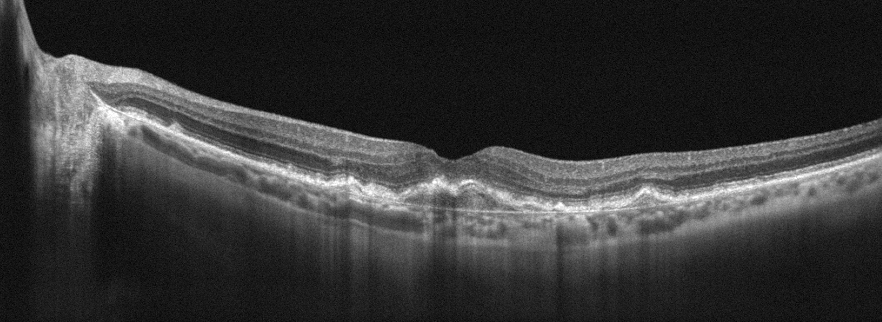
Retinal OCT cross-section; left eye; through the macula
The scan shows age-related macular degeneration.